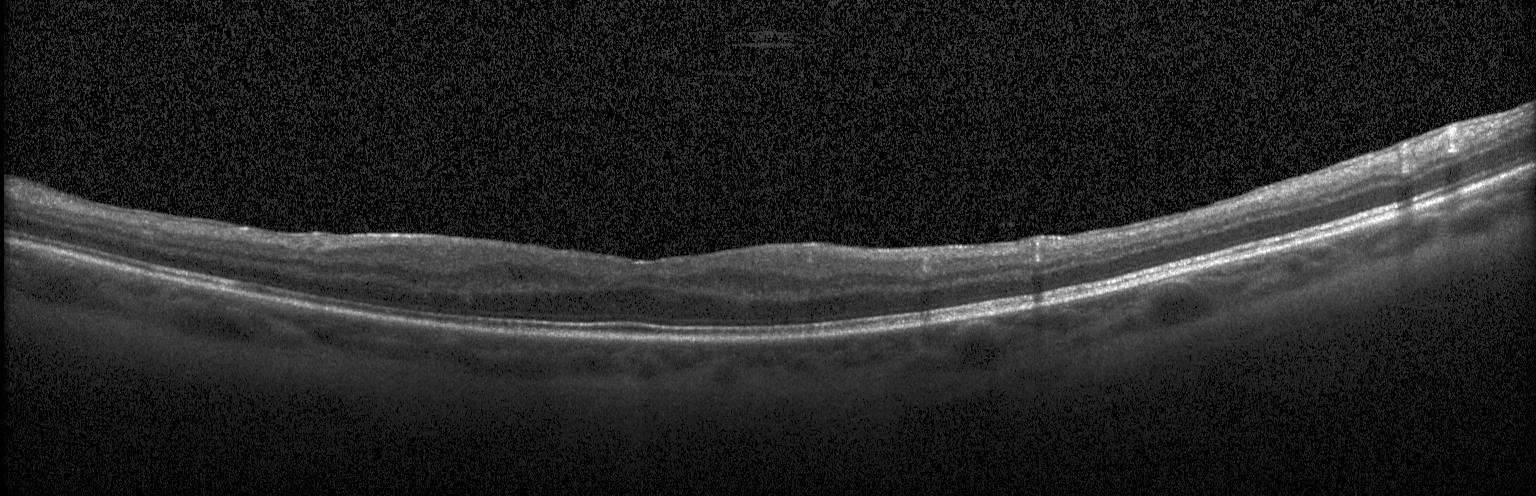 Spectral-domain optical coherence tomography. Optical coherence tomography scan — Macular OCT: diabetic macular edema.